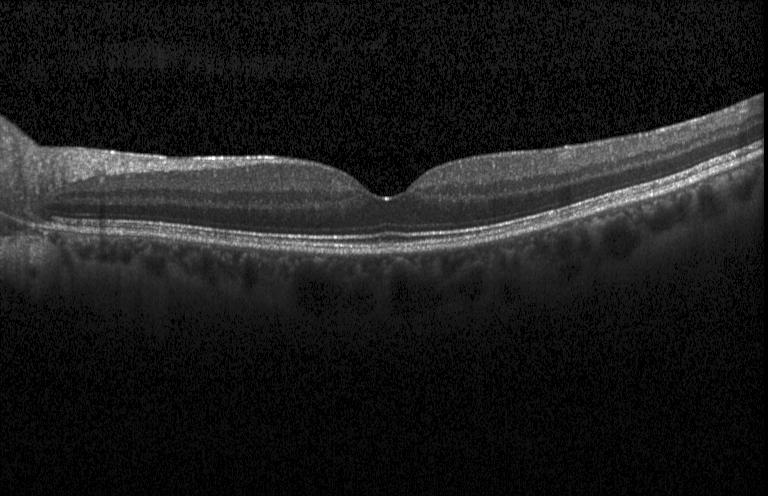
Acquired on a Heidelberg Spectralis; optical coherence tomography scan — Neither choroidal neovascularization, diabetic macular edema, nor drusen.